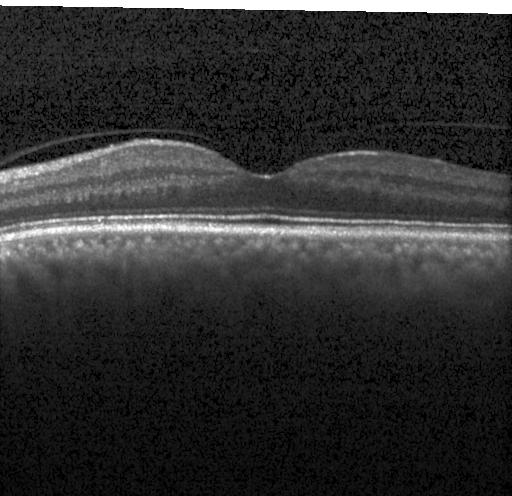 Retinal OCT cross-section.
Impression: no choroidal neovascularization, no diabetic macular edema, and no drusen.